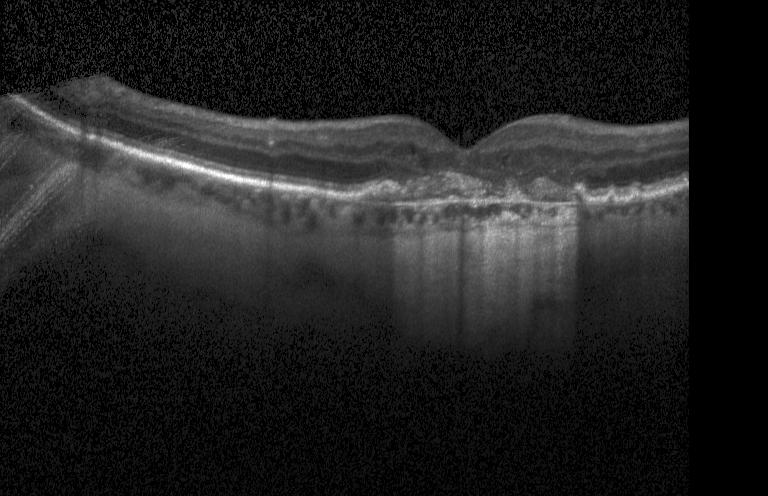
Choroidal neovascularization.